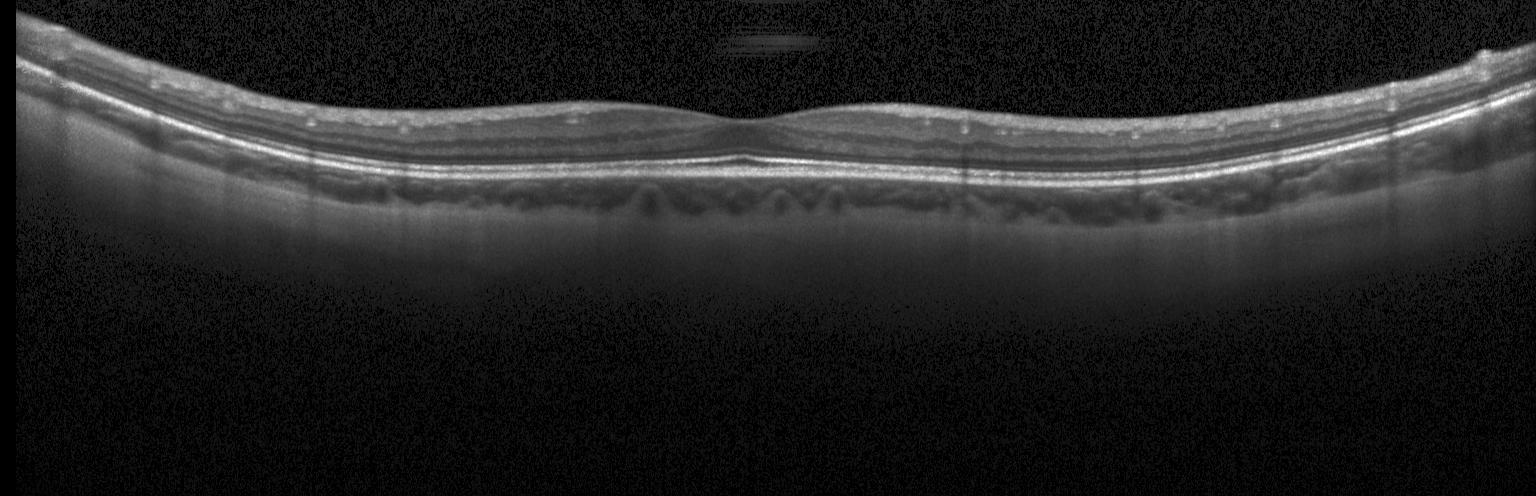 Retinal OCT cross-section, acquired on a Heidelberg Spectralis.
Finding: no evidence of choroidal neovascularization, diabetic macular edema, or drusen.